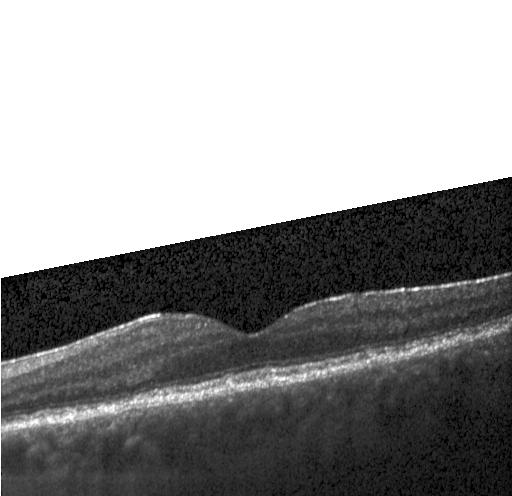

Impression: no CNV, no DME, and no drusen.